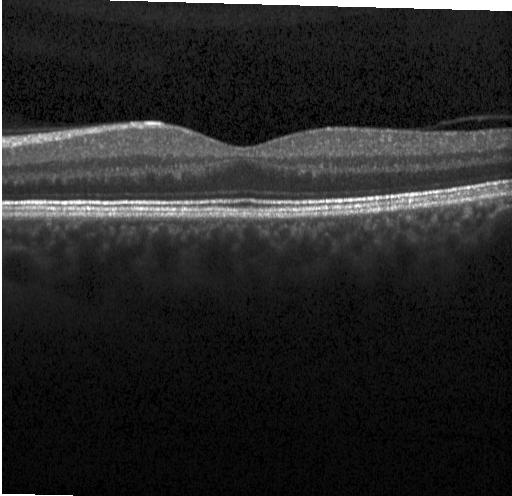 Finding: no evidence of choroidal neovascularization, diabetic macular edema, or drusen.